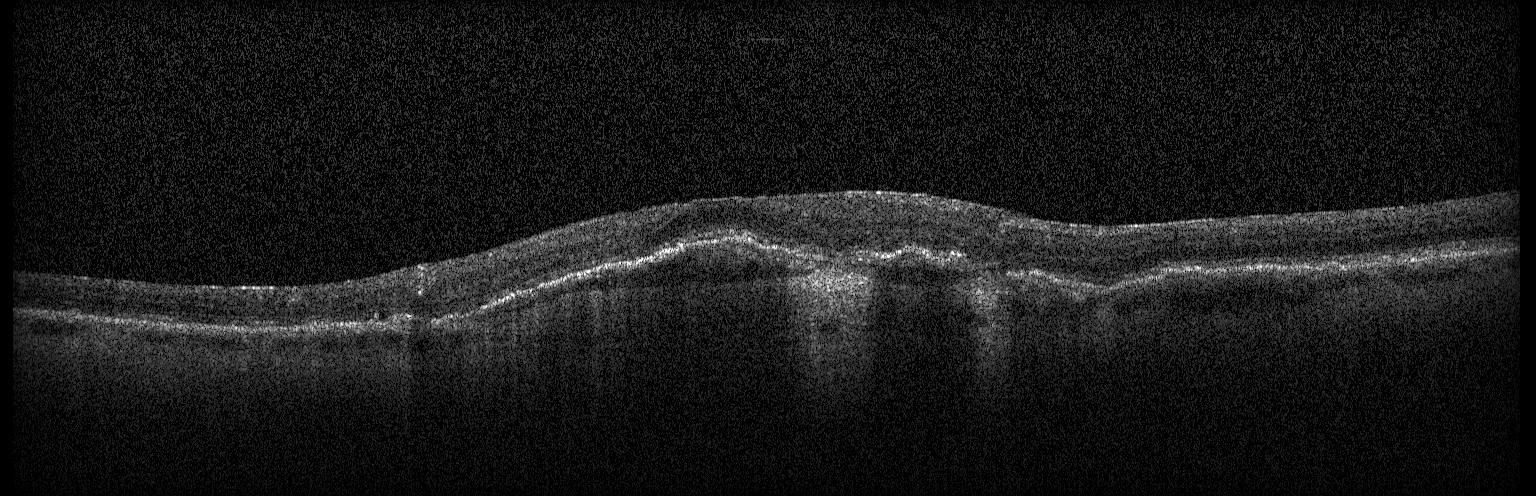 Assessment: choroidal neovascularization (CNV).